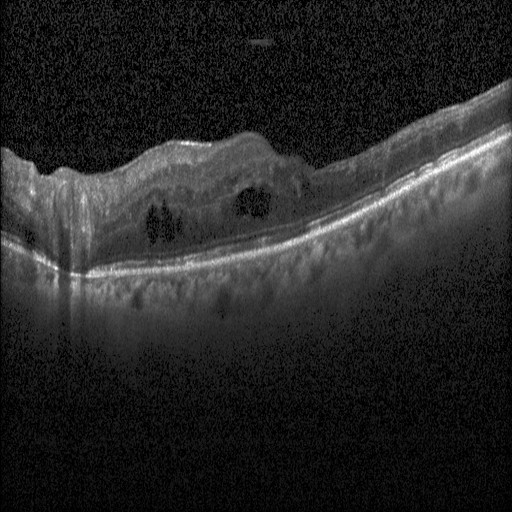 Optical coherence tomography B-scan. Spectral-domain optical coherence tomography. Fovea-centered — Finding: DME.